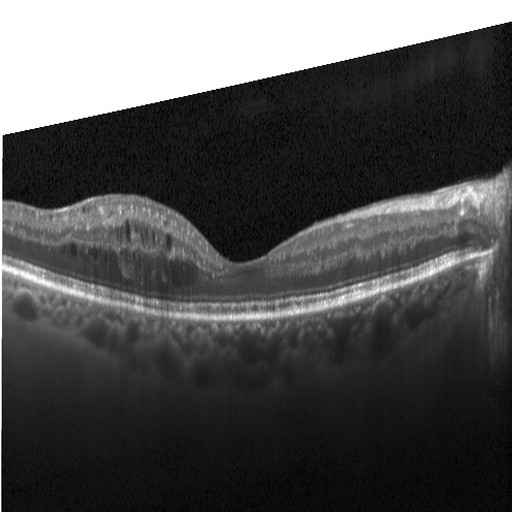 Optical coherence tomography B-scan. Acquired on a Heidelberg Spectralis — The scan shows DME.